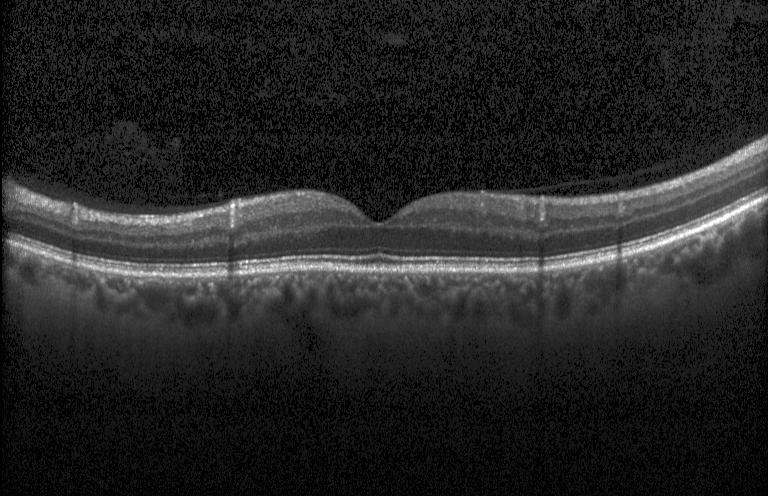
Retinal OCT cross-section. Impression: no evidence of CNV, DME, or drusen.